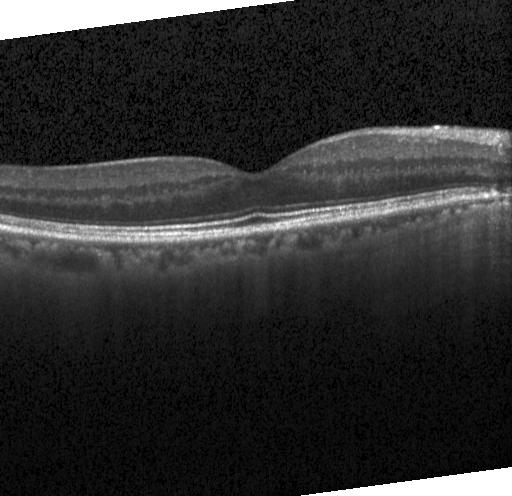
SD-OCT; centered on the fovea; retinal OCT cross-section
Macular OCT: no choroidal neovascularization, diabetic macular edema, or drusen.